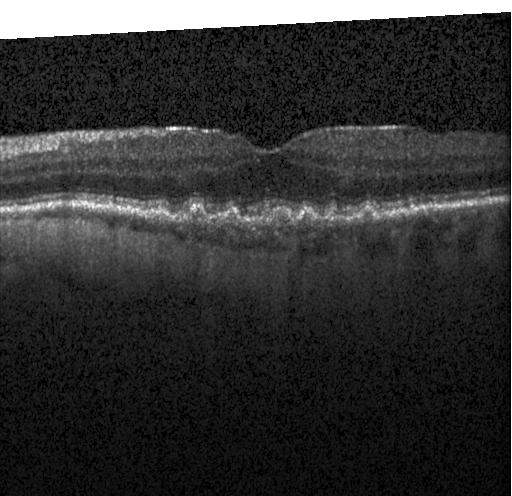

Optical coherence tomography B-scan; spectral-domain OCT; horizontal scan through the fovea.
The scan shows drusen.